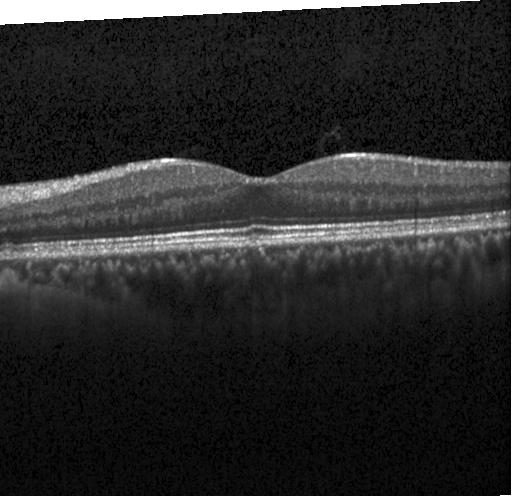
Retinal OCT cross-section — Dx: neither CNV, DME, nor drusen.